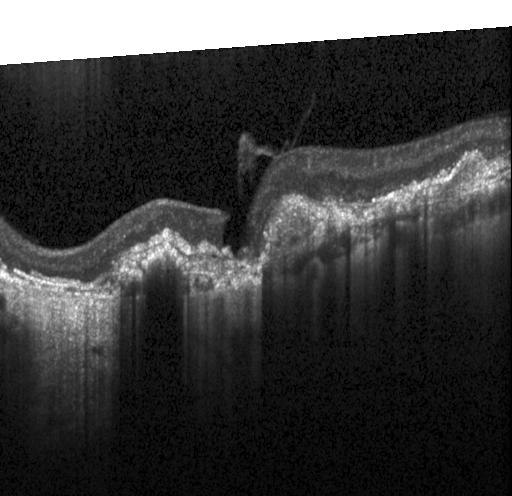 Optical coherence tomography scan
CNV.